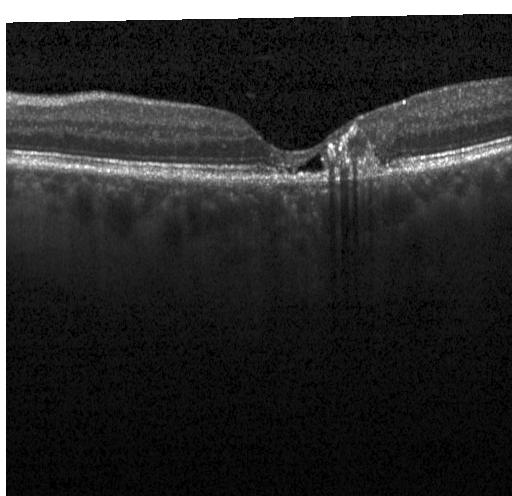 Heidelberg Spectralis. SD-OCT. Retinal OCT cross-section — Finding: a choroidal neovascular membrane.